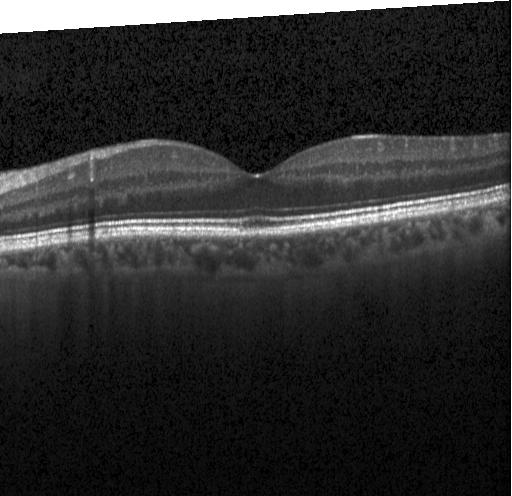

OCT B-scan.
Assessment: neither CNV, DME, nor drusen.